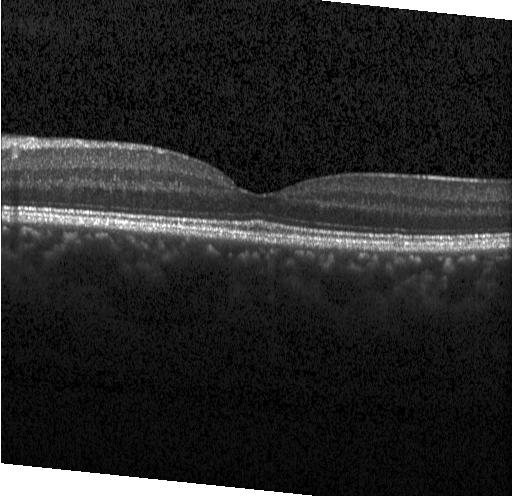
Impression: neither choroidal neovascularization, diabetic macular edema, nor drusen.